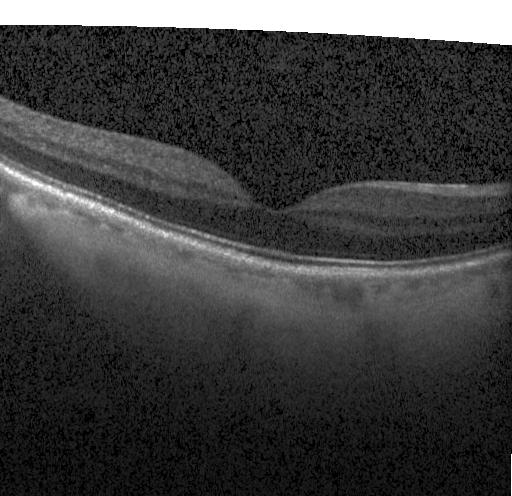 Acquired on a Heidelberg Spectralis, centered on the fovea, OCT B-scan, spectral-domain OCT.
Finding: neither choroidal neovascularization, diabetic macular edema, nor drusen.